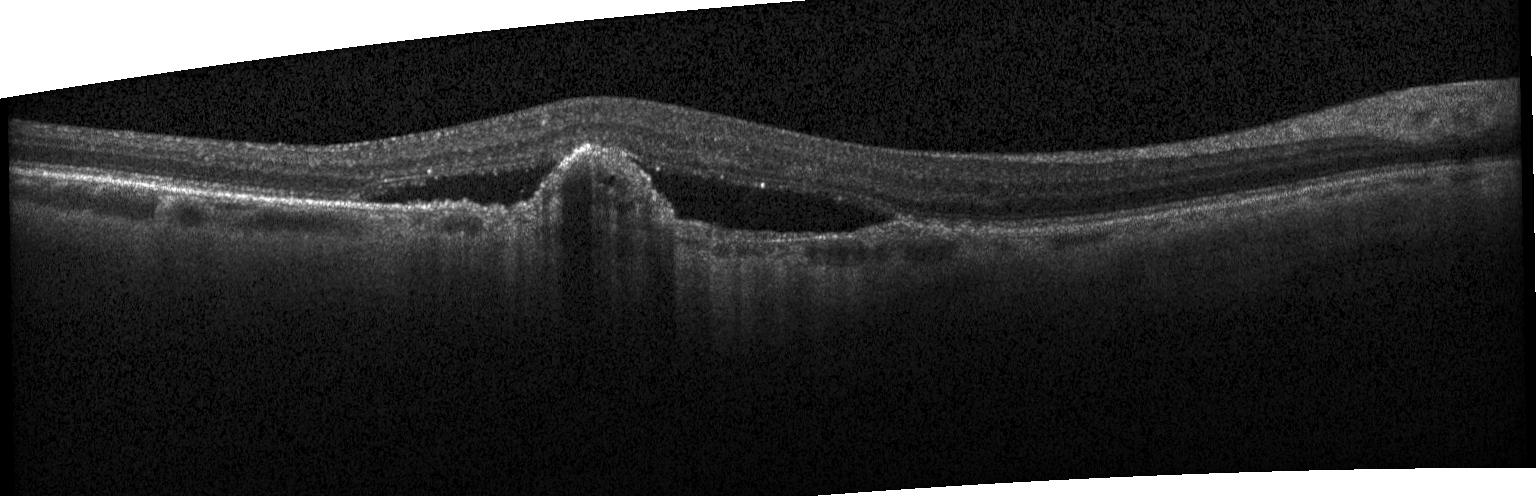

Impression: choroidal neovascularization.